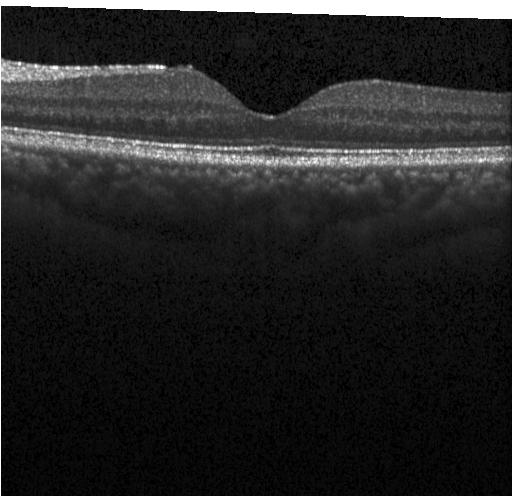 OCT line scan; horizontal scan through the fovea; acquired on a Heidelberg Spectralis. Dx: neither CNV, DME, nor drusen.